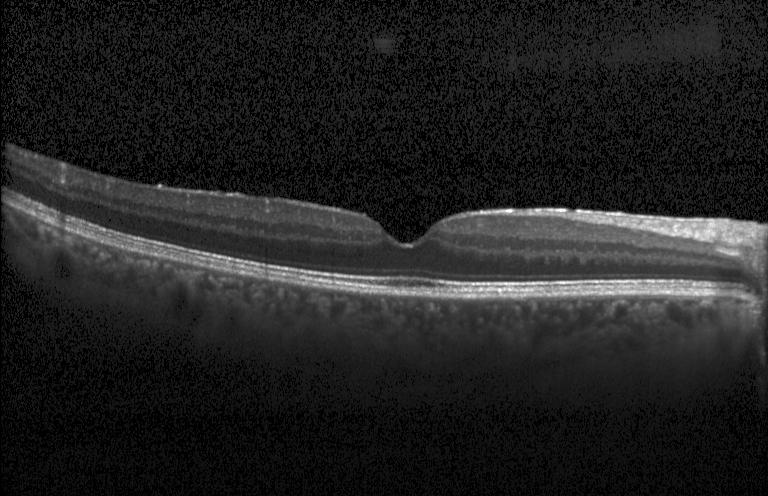
Retinal OCT B-scan
Assessment: neither CNV, DME, nor drusen.